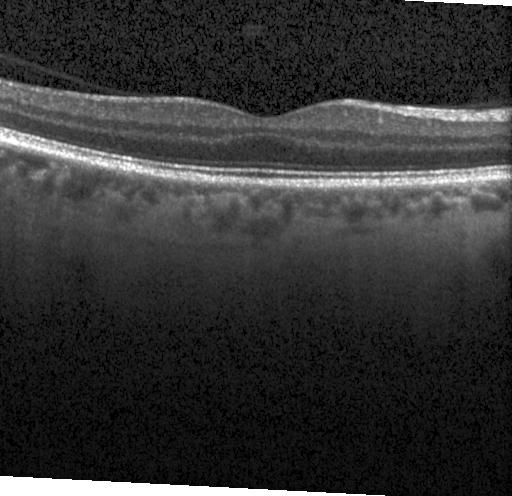

Dx: neither CNV, DME, nor drusen.